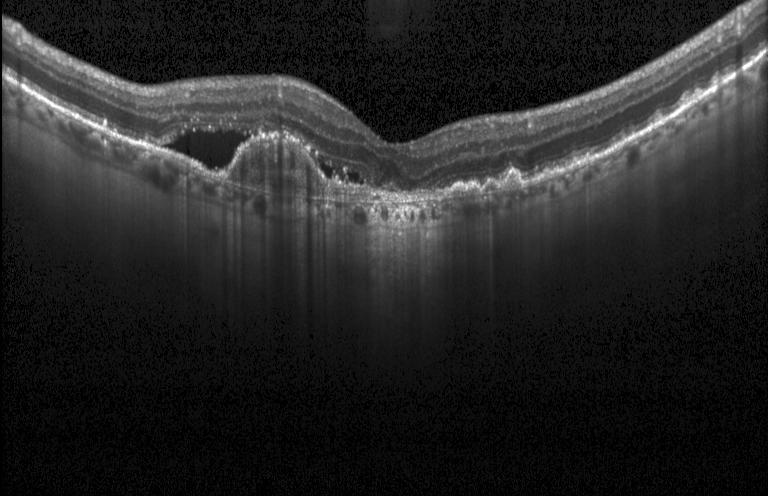
OCT line scan. Impression: choroidal neovascularization.